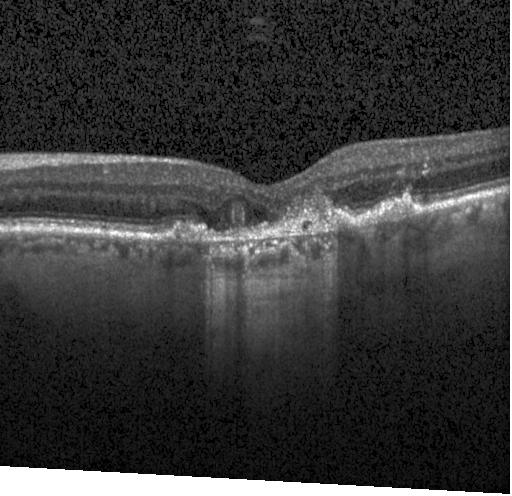

SD-OCT; optical coherence tomography B-scan
Macular OCT: a choroidal neovascular membrane.